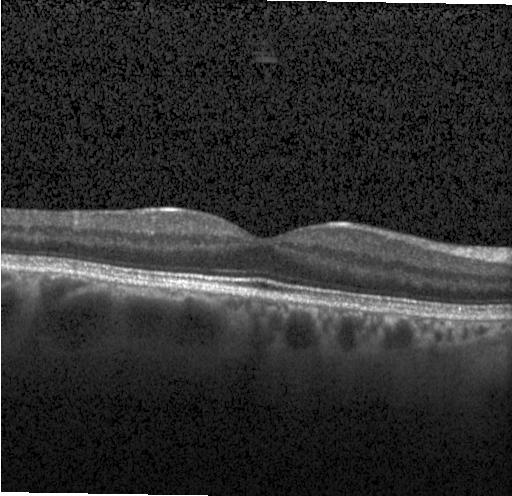

Heidelberg Spectralis; optical coherence tomography B-scan
Finding: no choroidal neovascularization, no diabetic macular edema, and no drusen.